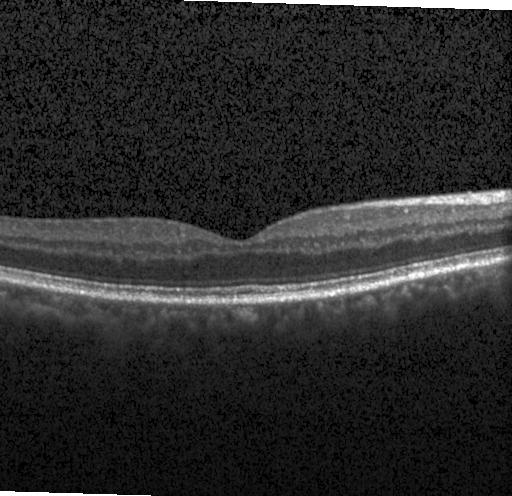 Heidelberg Spectralis, spectral-domain OCT, optical coherence tomography scan
Impression: no CNV, no DME, and no drusen.